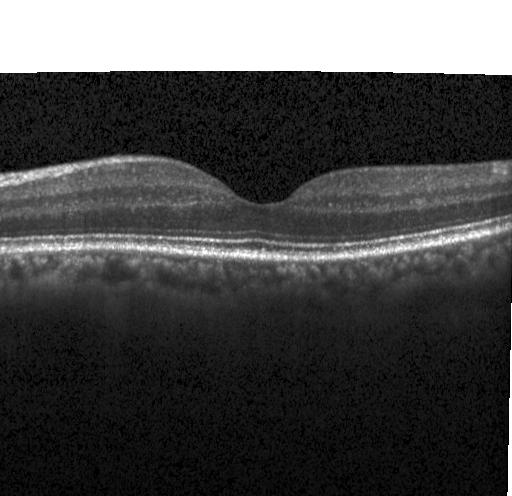
Optical coherence tomography scan. Through the macula.
OCT finding: no choroidal neovascularization, no diabetic macular edema, and no drusen.